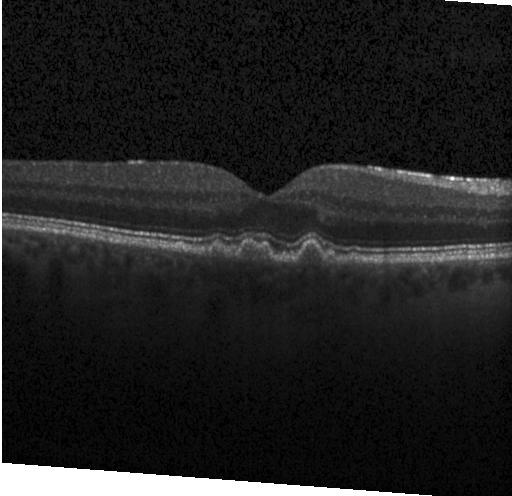

Retinal OCT B-scan · Heidelberg Spectralis OCT system — Impression: sub-RPE drusenoid deposits.